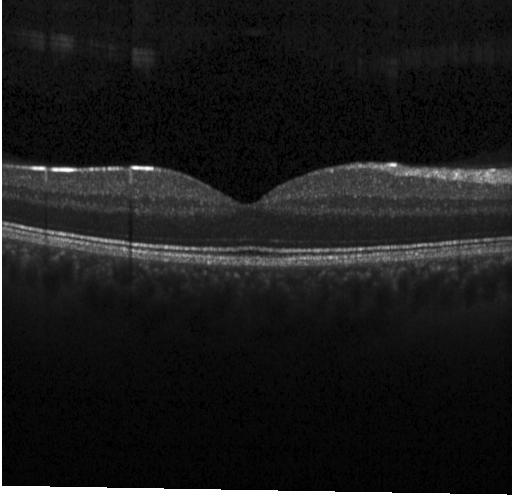

The scan shows neither choroidal neovascularization, diabetic macular edema, nor drusen.